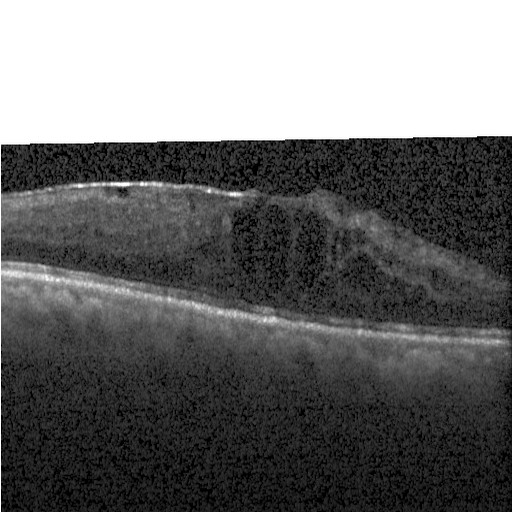
Optical coherence tomography B-scan
This B-scan demonstrates diabetic macular edema.